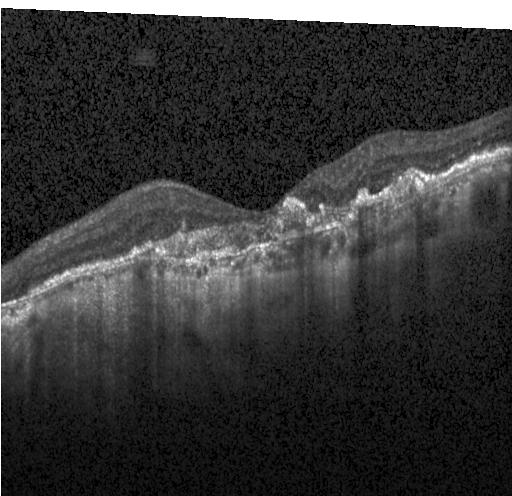
Finding: choroidal neovascularization.